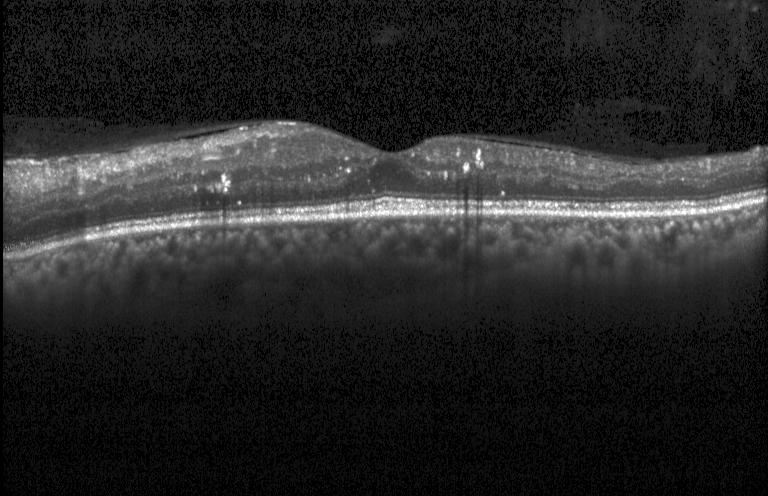
The scan shows diabetic macular edema.